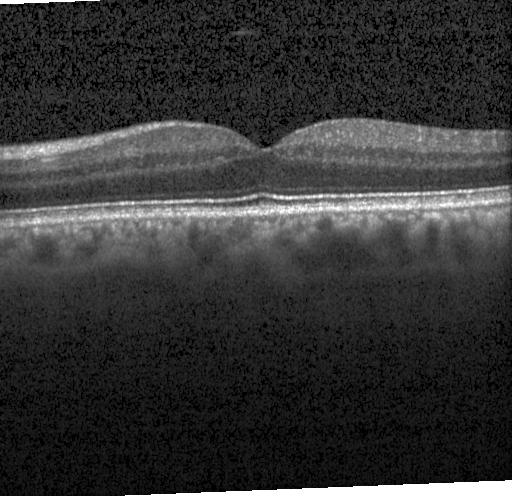 Optical coherence tomography scan. Heidelberg Spectralis. Through the macula.
Impression: neither choroidal neovascularization, diabetic macular edema, nor drusen.